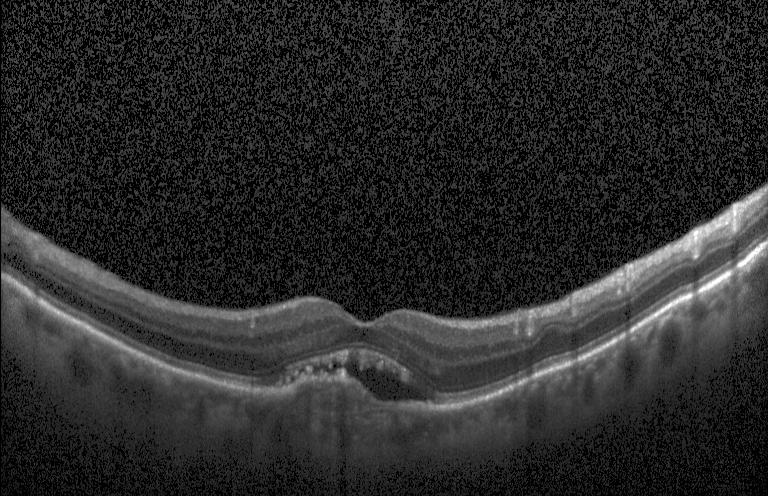
Optical coherence tomography B-scan — Impression: choroidal neovascularization (CNV).